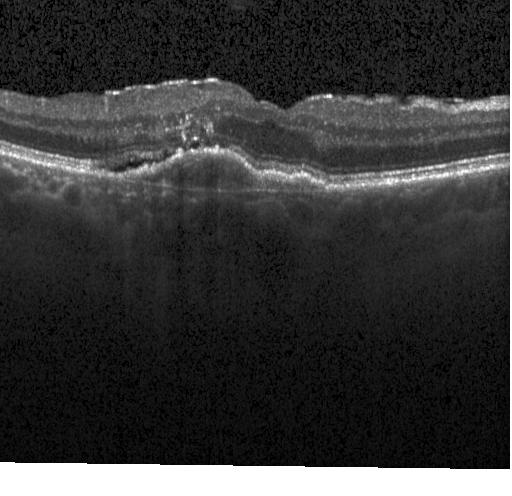

Finding: choroidal neovascularization.